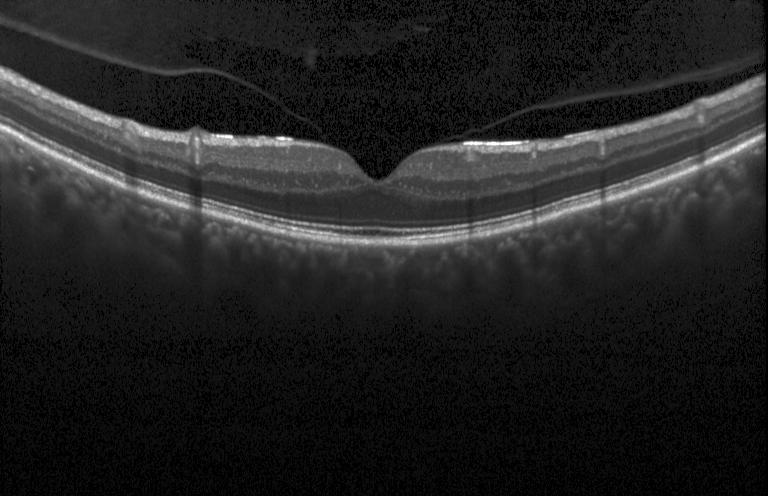

Heidelberg Spectralis OCT system · SD-OCT · horizontal scan through the fovea · retinal OCT cross-section
Diagnosis: neither choroidal neovascularization, diabetic macular edema, nor drusen.